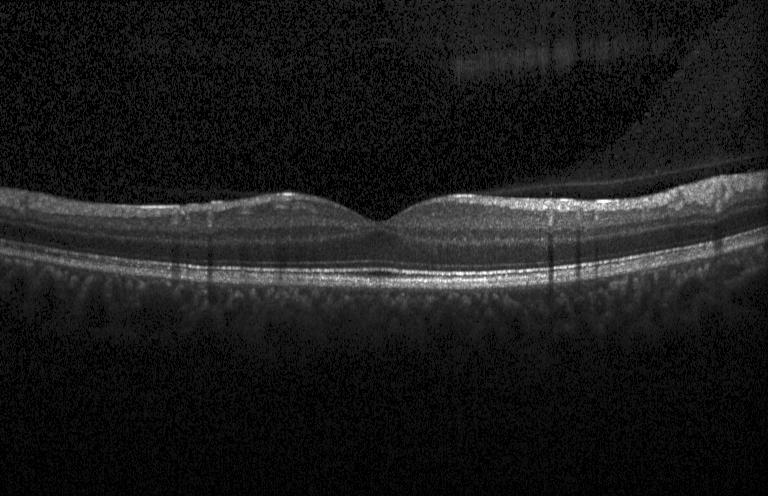

Macular OCT demonstrating no CNV, DME, or drusen.